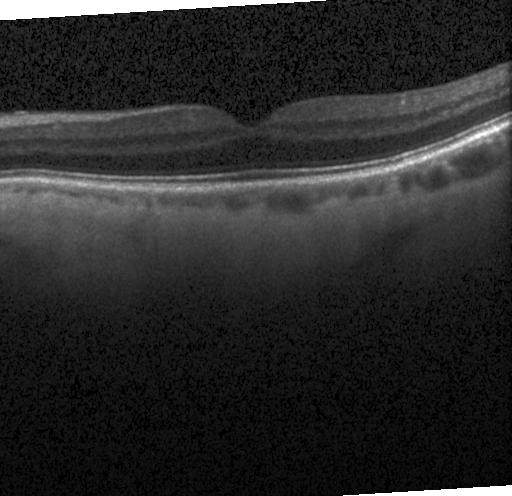 OCT line scan — Assessment: no CNV, DME, or drusen.